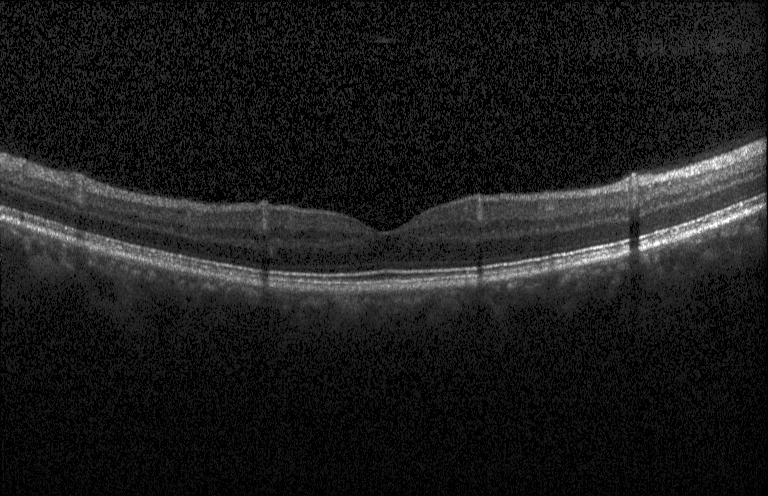

Finding: no choroidal neovascularization, diabetic macular edema, or drusen.